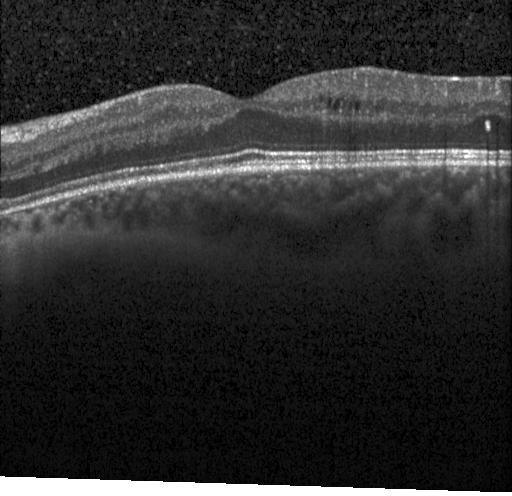

SD-OCT · acquired on a Heidelberg Spectralis · horizontal scan through the fovea · retinal OCT B-scan
Impression: diabetic macular edema (DME).